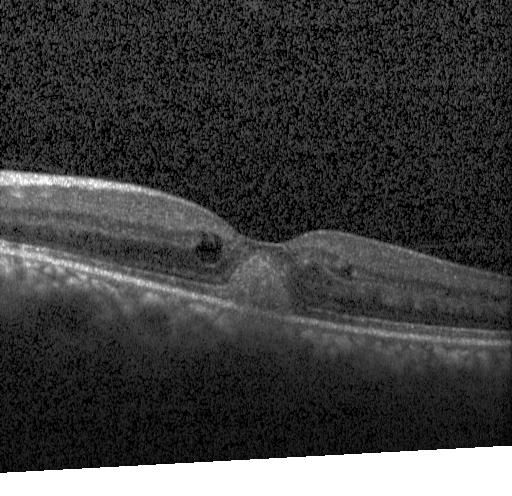

Spectral-domain optical coherence tomography · optical coherence tomography scan.
Choroidal neovascularization.